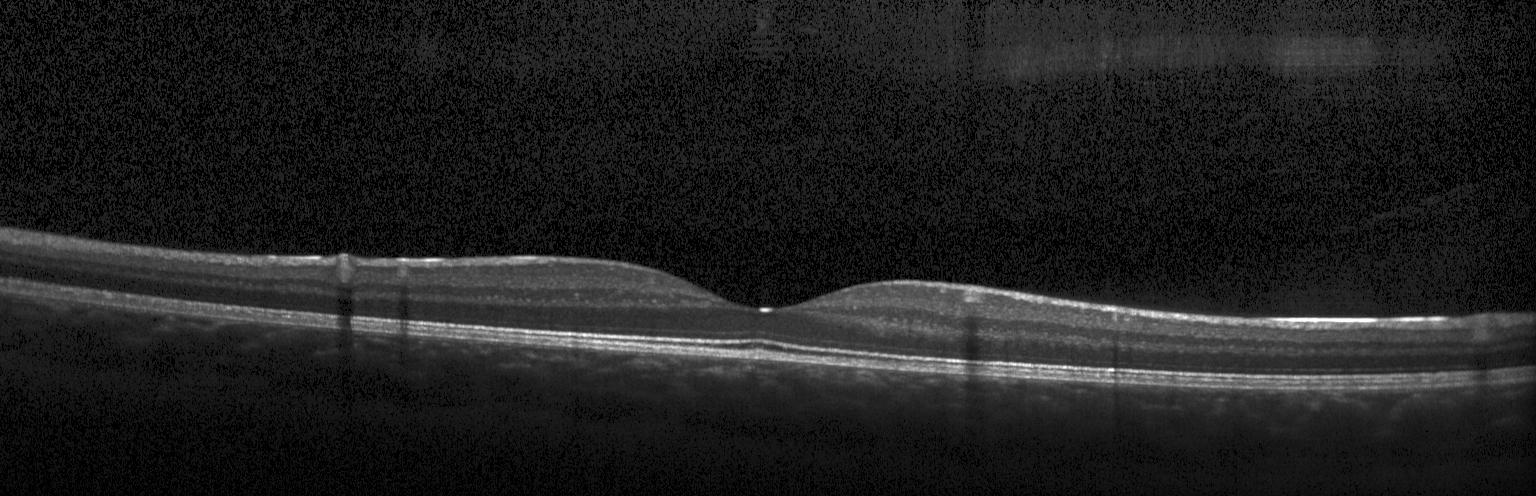

OCT B-scan. Diagnosis: neither choroidal neovascularization, diabetic macular edema, nor drusen.